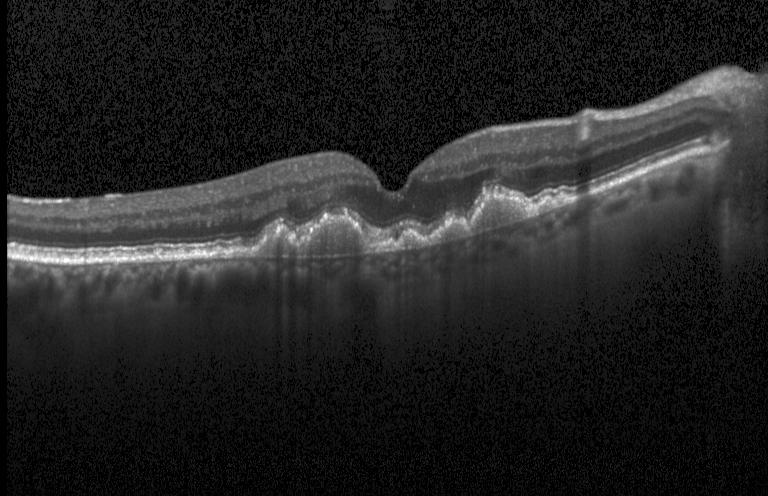
Optical coherence tomography scan, through the macula, spectral-domain OCT, Heidelberg Spectralis. Impression: sub-RPE drusenoid deposits.